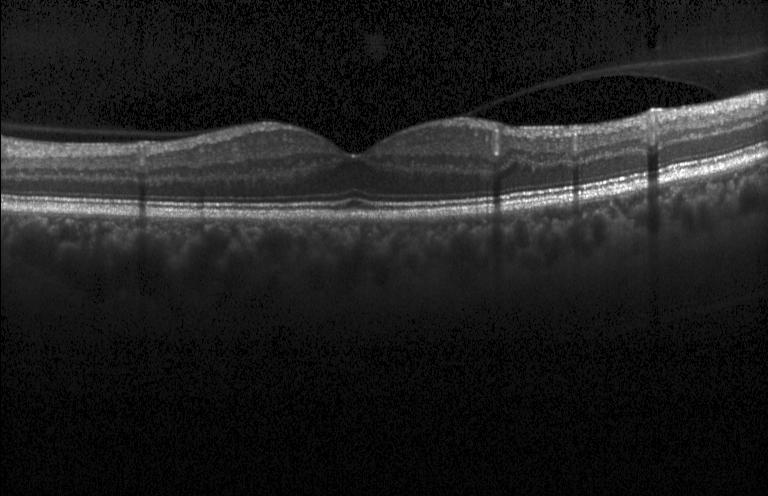 The scan shows no choroidal neovascularization, diabetic macular edema, or drusen.